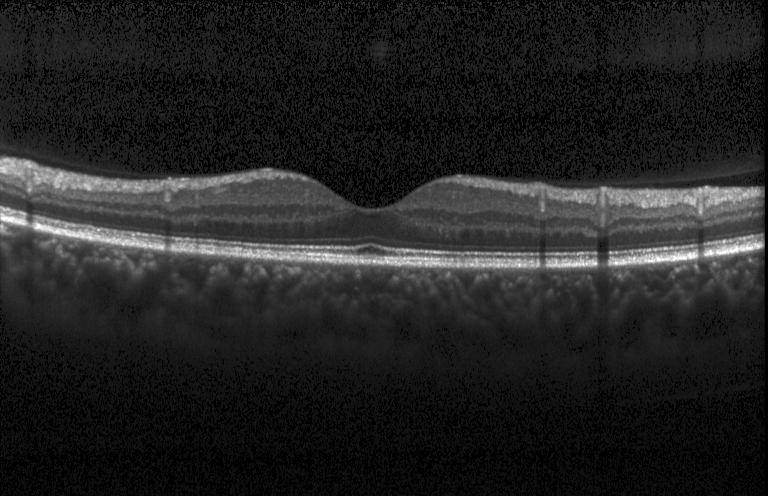 The scan shows no choroidal neovascularization, no diabetic macular edema, and no drusen.